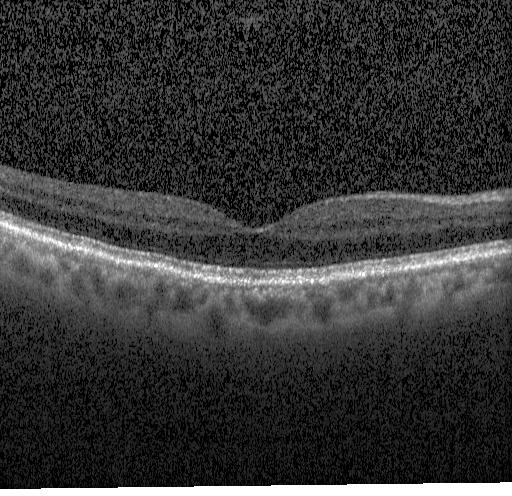
Spectral-domain OCT B-scan: neither choroidal neovascularization, diabetic macular edema, nor drusen.